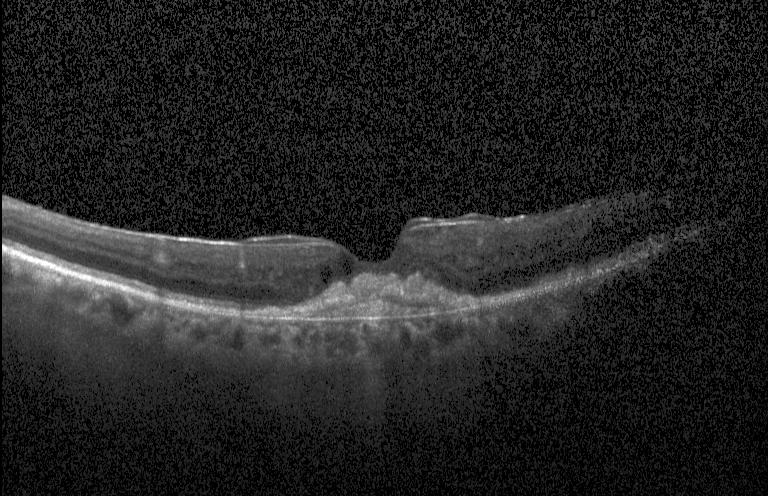

Retinal OCT B-scan. Impression: a choroidal neovascular membrane.